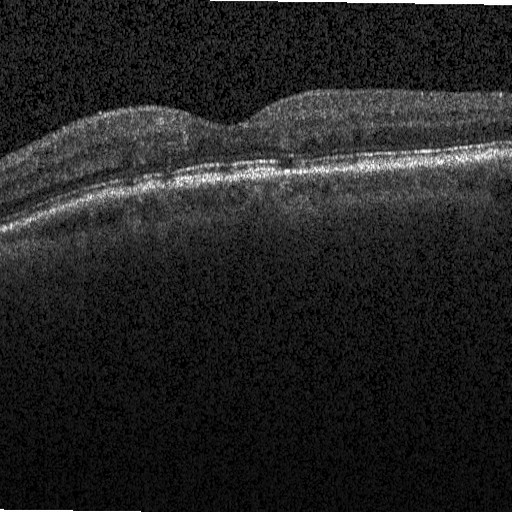
SD-OCT, macular scan, retinal OCT B-scan. This B-scan demonstrates diabetic macular edema (DME).